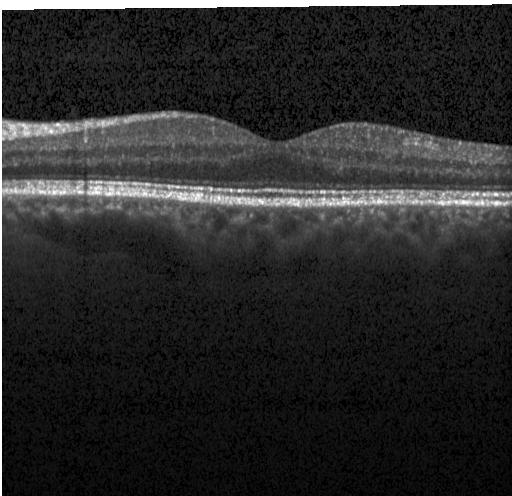
Spectral-domain optical coherence tomography; optical coherence tomography scan; horizontal scan through the fovea — Diagnosis: no choroidal neovascularization, no diabetic macular edema, and no drusen.